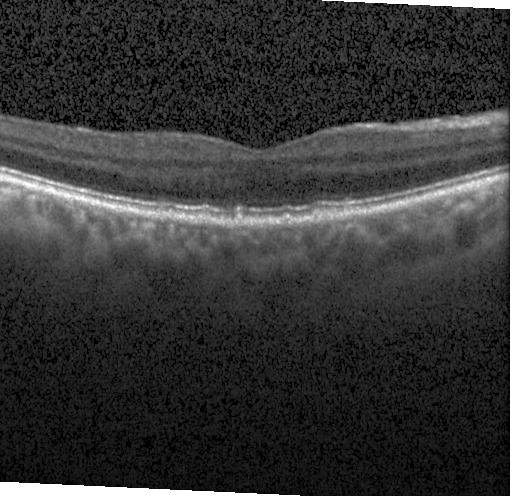
Finding: drusen.